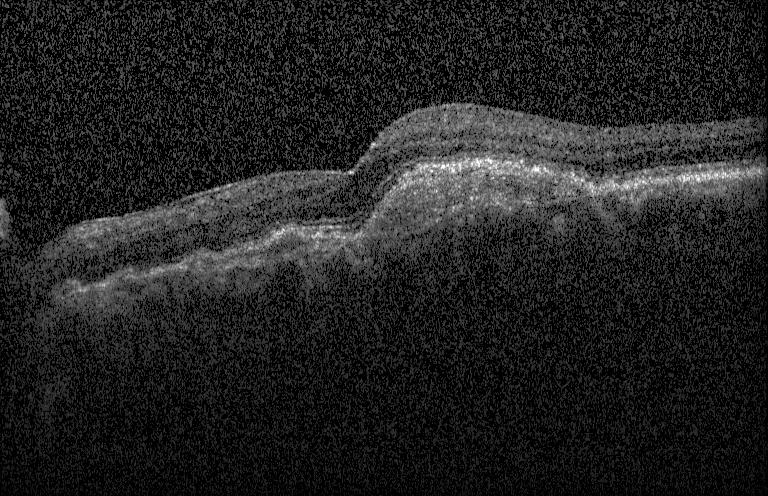 OCT B-scan.
Macular OCT: CNV.